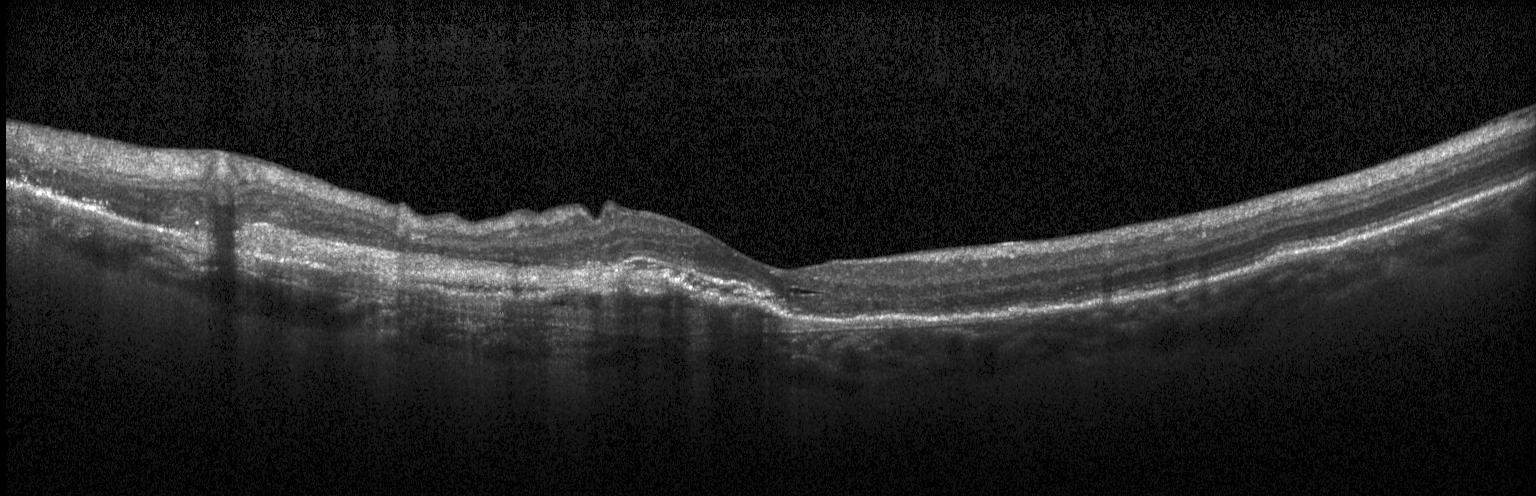
The scan shows CNV.